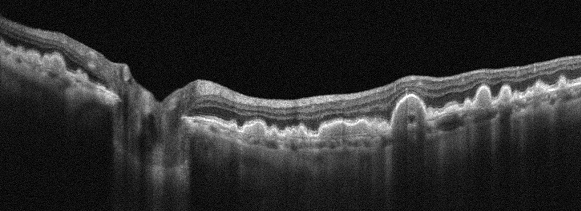 Optical coherence tomography scan
Diagnosis: age-related macular degeneration (AMD).